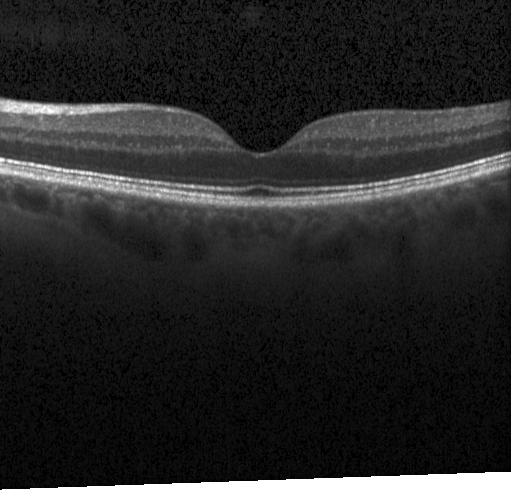
Heidelberg Spectralis. OCT line scan. Spectral-domain optical coherence tomography. Centered on the fovea. Finding: no choroidal neovascularization, no diabetic macular edema, and no drusen.